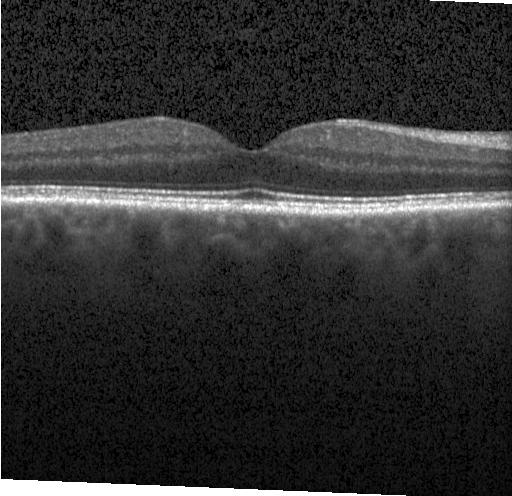
Impression: no choroidal neovascularization, diabetic macular edema, or drusen.